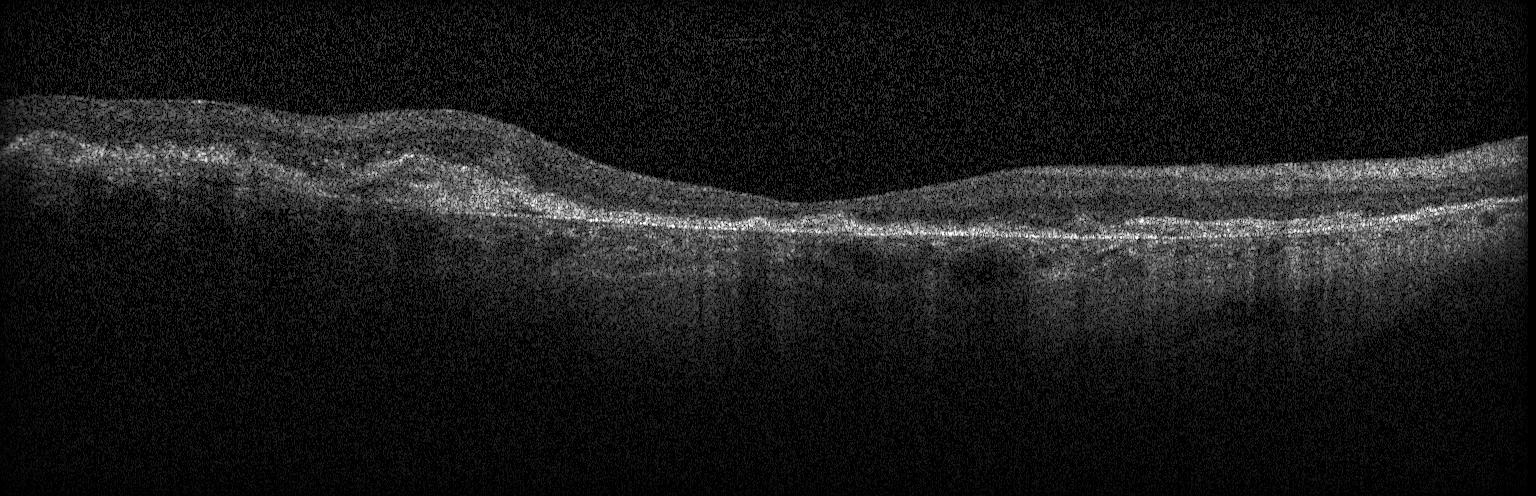
OCT B-scan. SD-OCT. Finding: a choroidal neovascular membrane.